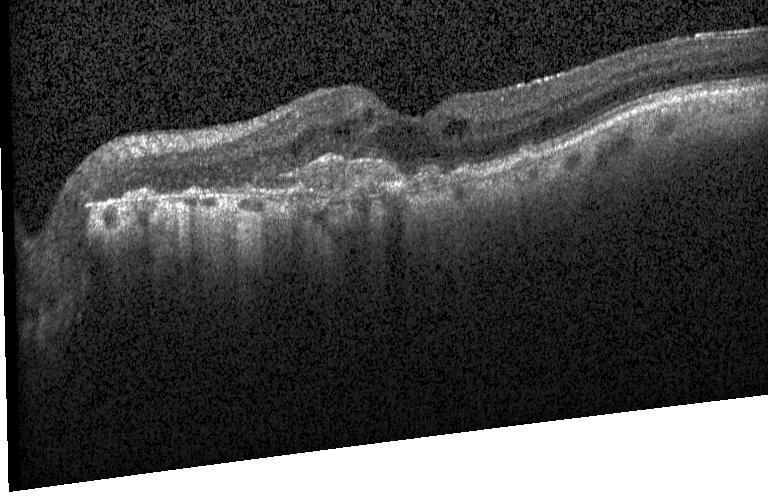 Finding: choroidal neovascularization (CNV).